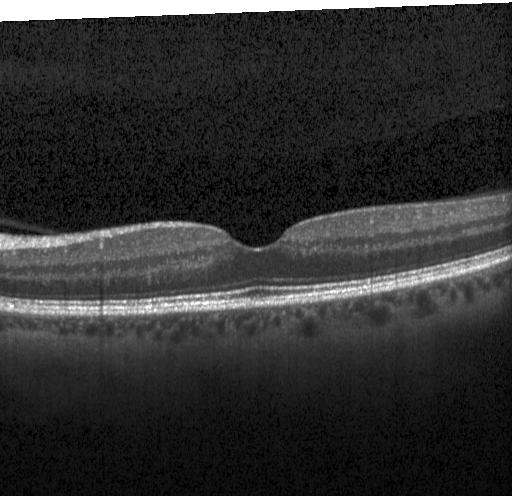
Optical coherence tomography scan
Dx: no evidence of choroidal neovascularization, diabetic macular edema, or drusen.